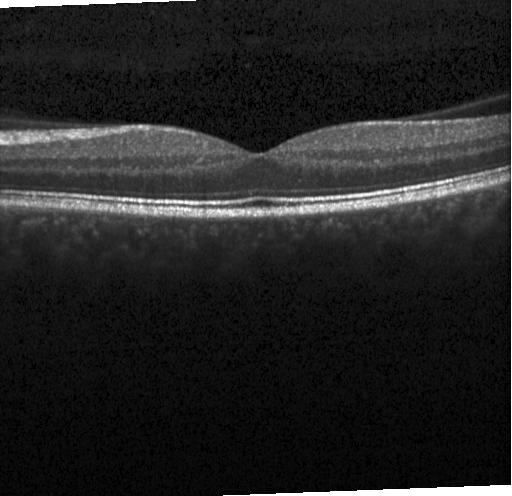 Spectral-domain OCT B-scan: neither CNV, DME, nor drusen.